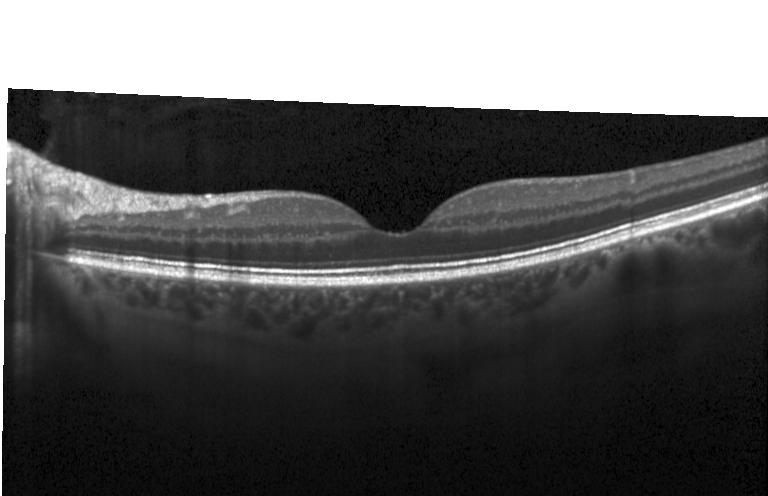

Optical coherence tomography scan
Dx: neither choroidal neovascularization, diabetic macular edema, nor drusen.